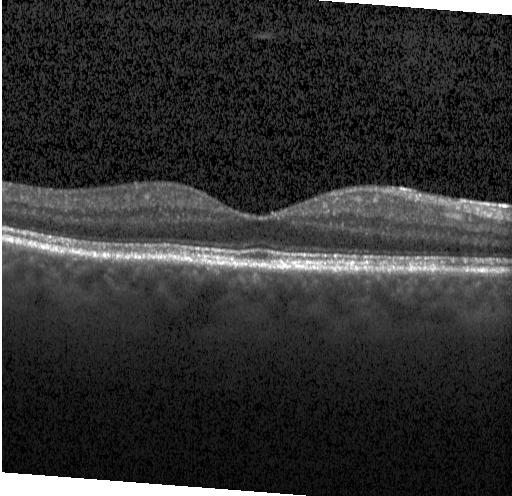
Retinal OCT B-scan
Assessment: no CNV, no DME, and no drusen.